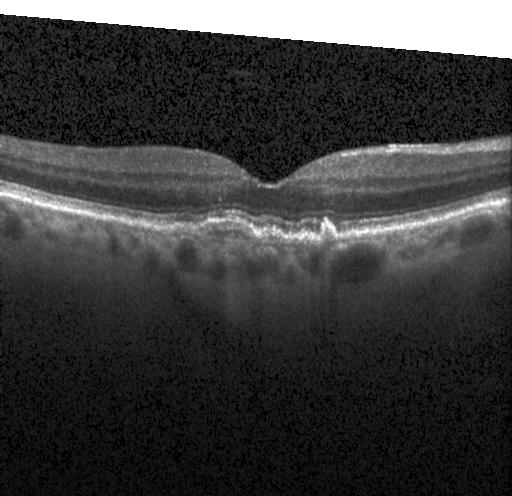
Spectral-domain OCT · retinal OCT B-scan · fovea-centered · instrument: Heidelberg Spectralis
Choroidal neovascularization.